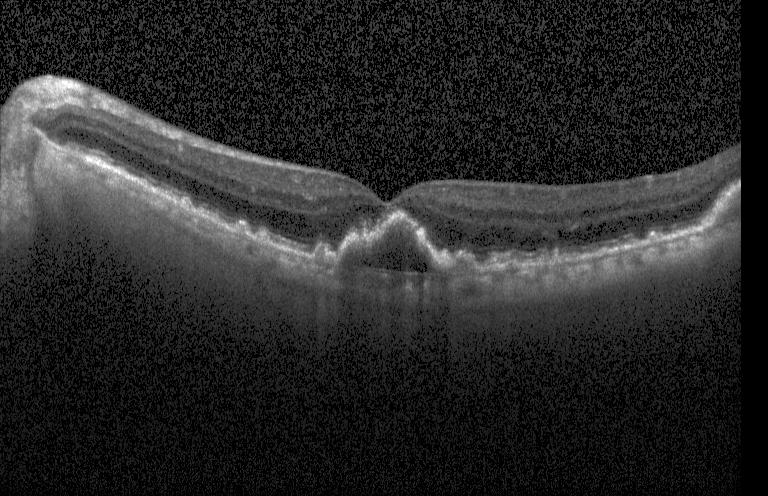

Finding: a choroidal neovascular membrane.